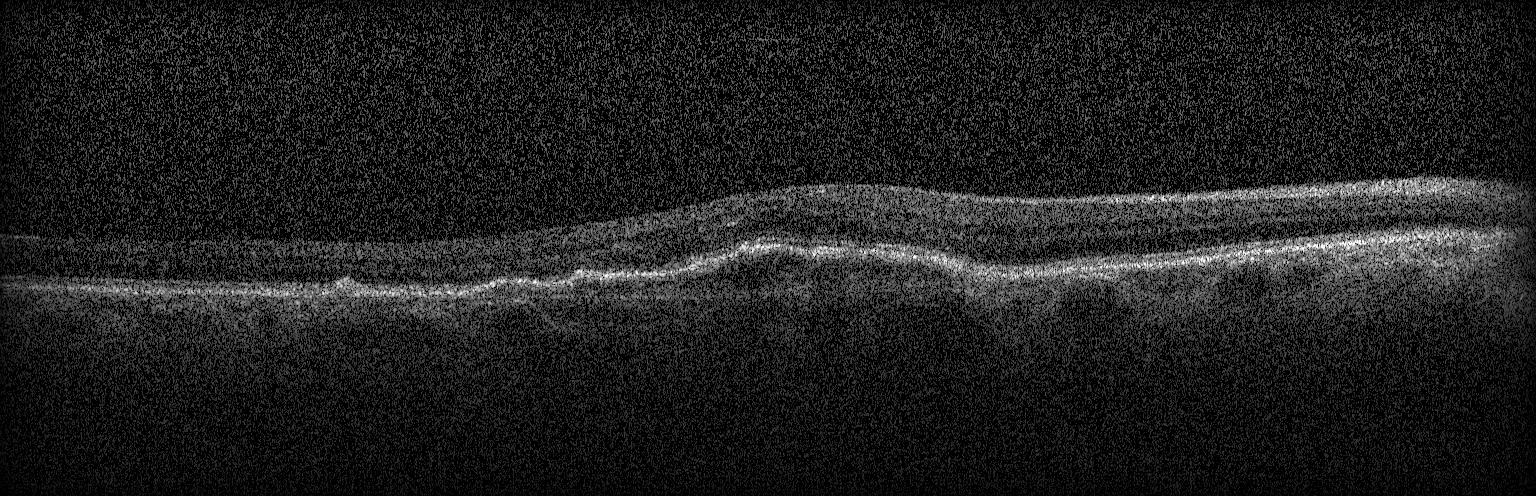
Centered on the fovea, Heidelberg Spectralis, optical coherence tomography B-scan, spectral-domain OCT.
Diagnosis: CNV.